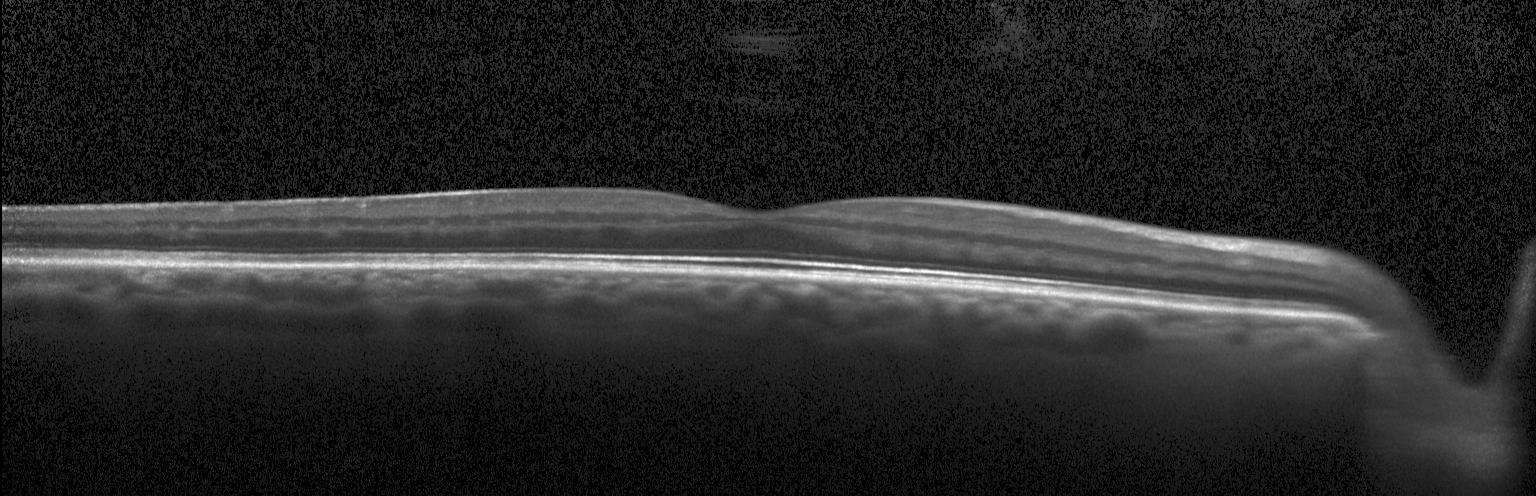
SD-OCT · retinal OCT B-scan · instrument: Heidelberg Spectralis · centered on the fovea. The scan shows no CNV, DME, or drusen.